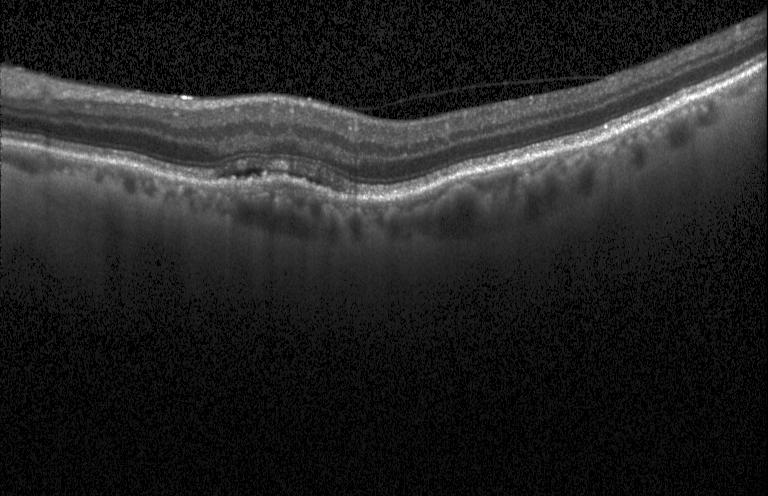

Macular OCT: a choroidal neovascular membrane.